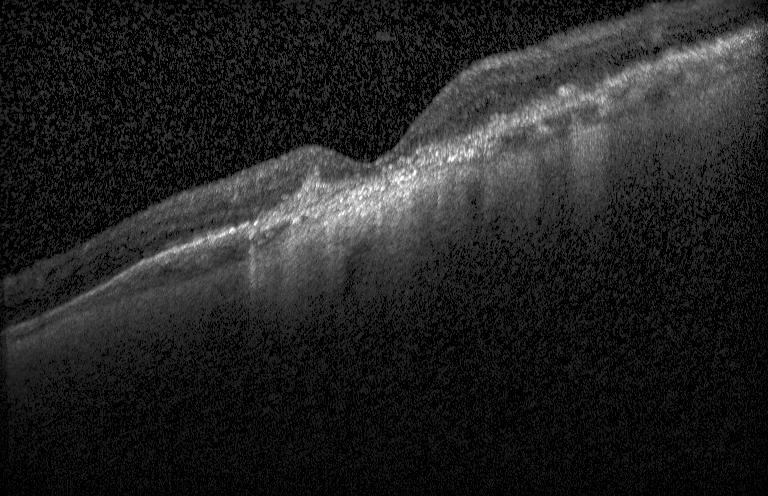
Optical coherence tomography B-scan · spectral-domain OCT · instrument: Heidelberg Spectralis · centered on the fovea.
Macular OCT: a choroidal neovascular membrane.